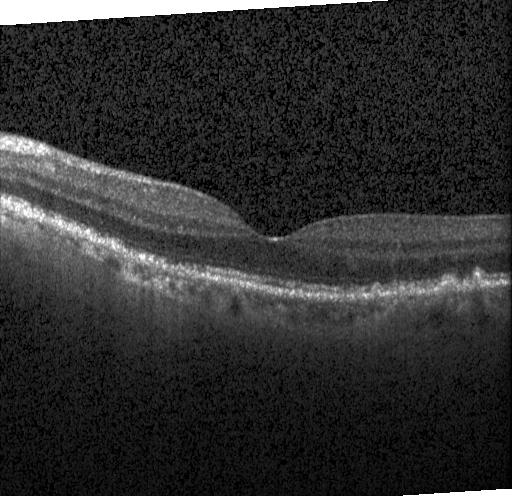

Diagnosis: sub-RPE drusenoid deposits.